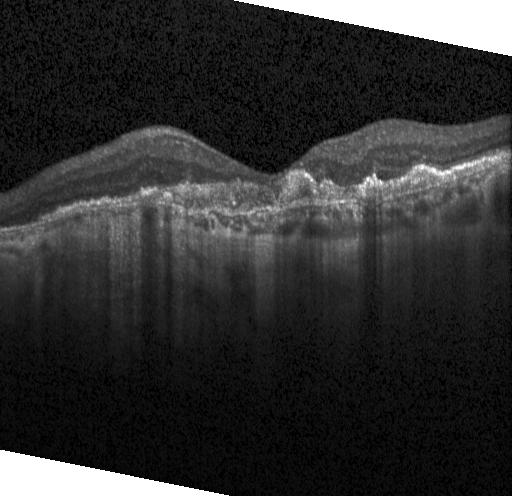

Instrument: Heidelberg Spectralis. SD-OCT. Optical coherence tomography B-scan. Fovea-centered
Finding: choroidal neovascularization.